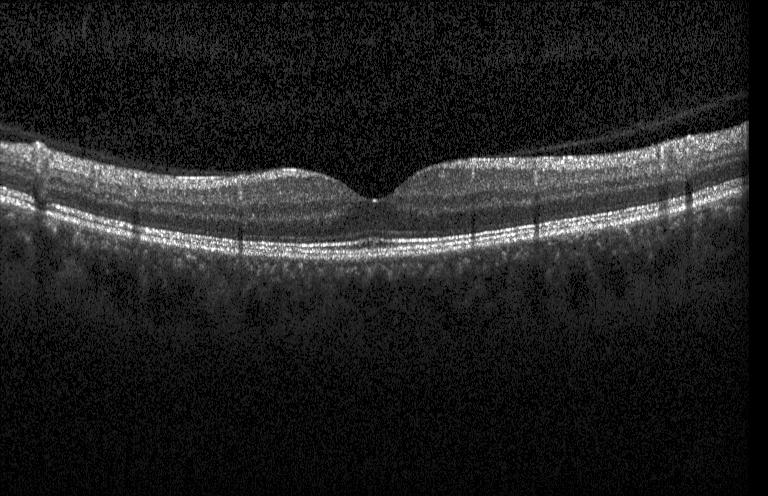 Acquired on a Heidelberg Spectralis. Retinal OCT B-scan. SD-OCT. Fovea-centered. Macular OCT: no choroidal neovascularization, no diabetic macular edema, and no drusen.